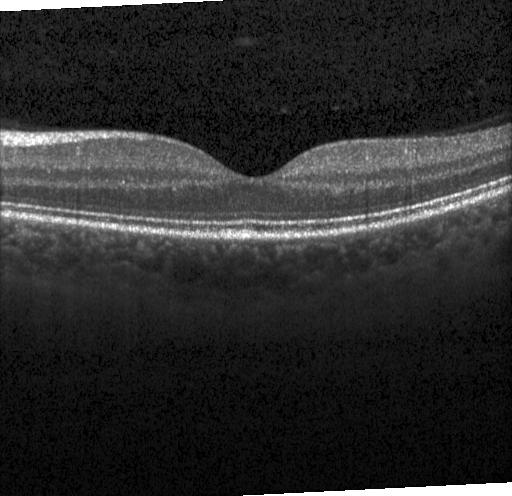
Spectral-domain optical coherence tomography; horizontal scan through the fovea; Heidelberg Spectralis; optical coherence tomography scan. Diagnosis: no choroidal neovascularization, no diabetic macular edema, and no drusen.